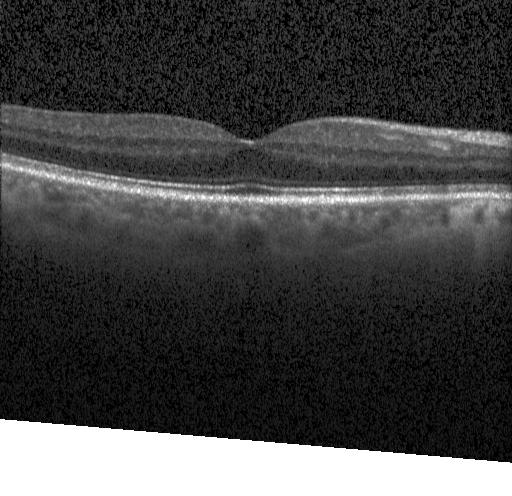 Horizontal scan through the fovea; Heidelberg Spectralis; retinal OCT B-scan
This B-scan demonstrates no choroidal neovascularization, no diabetic macular edema, and no drusen.